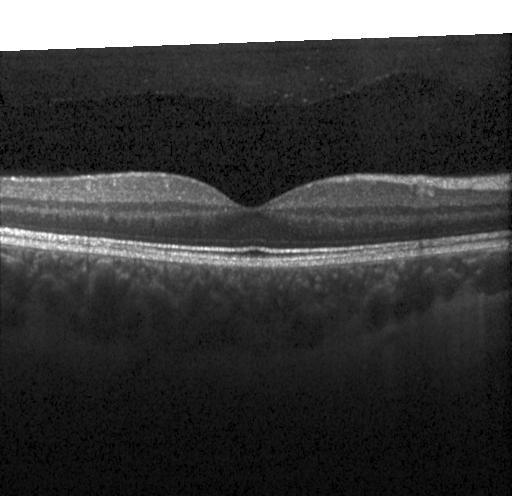

Diagnosis: no CNV, DME, or drusen.